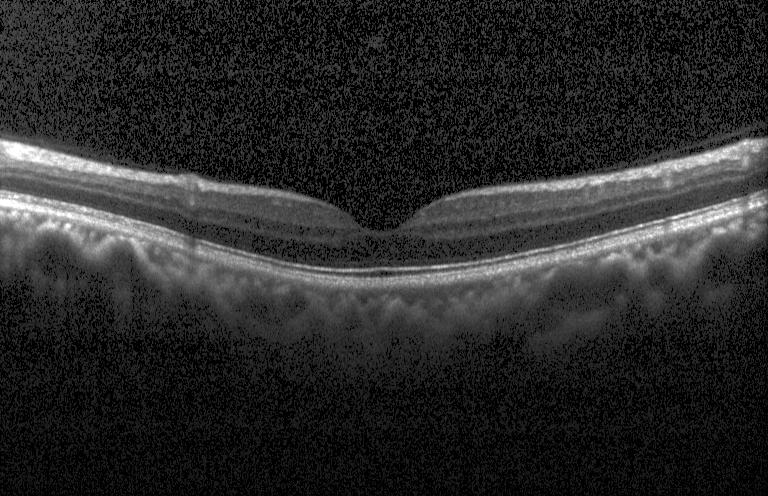
Heidelberg Spectralis. OCT B-scan. Spectral-domain optical coherence tomography. Macular scan. Dx: no CNV, no DME, and no drusen.